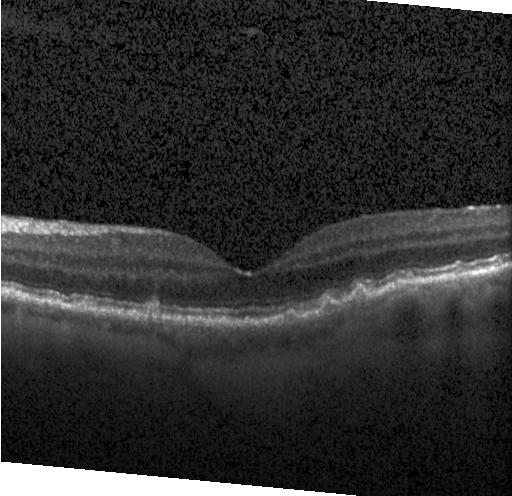
Diagnosis: multiple drusen.